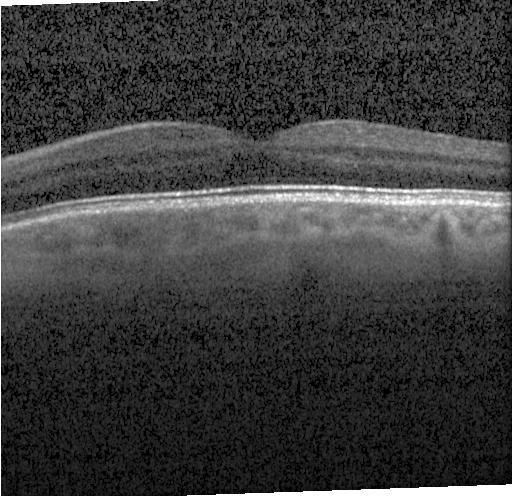
Finding: no choroidal neovascularization, diabetic macular edema, or drusen.